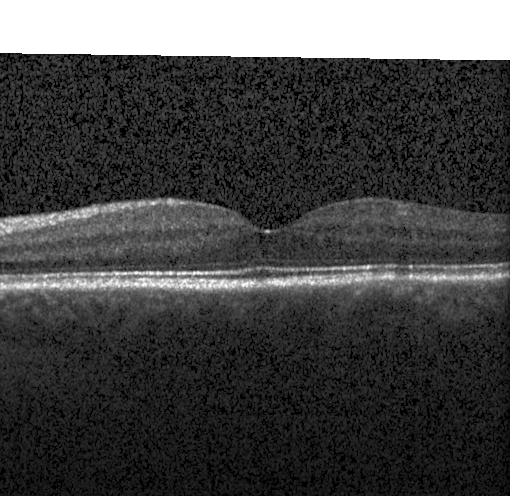 Through the macula, instrument: Heidelberg Spectralis, optical coherence tomography B-scan.
Impression: no CNV, no DME, and no drusen.